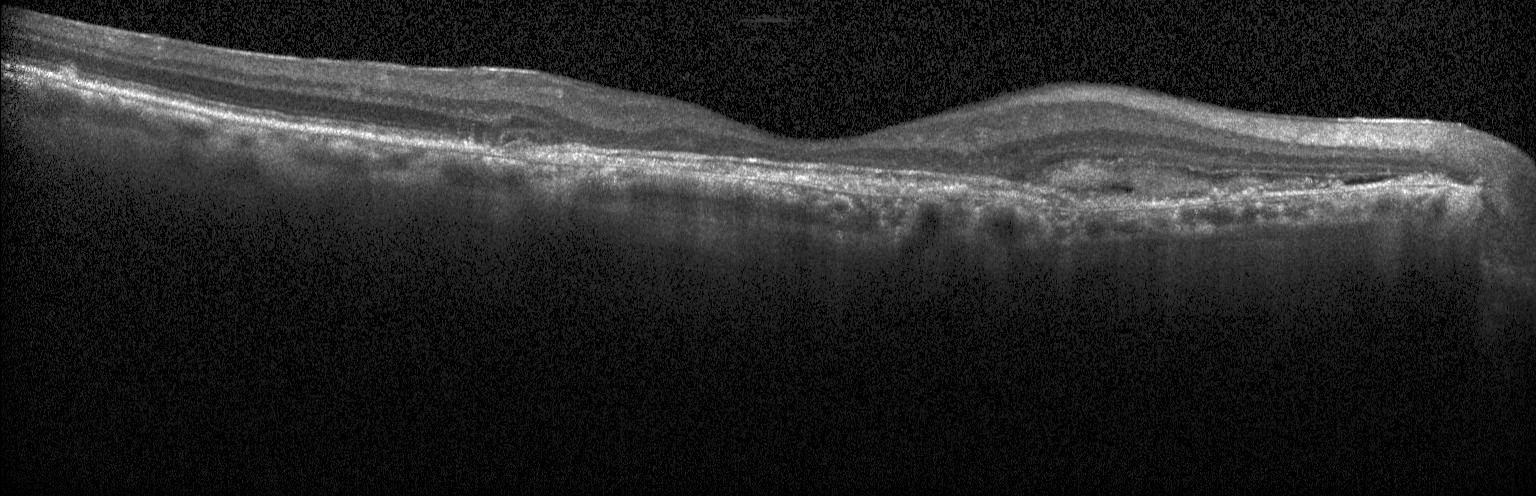
Spectral-domain OCT. Retinal OCT cross-section — This B-scan demonstrates a choroidal neovascular membrane.